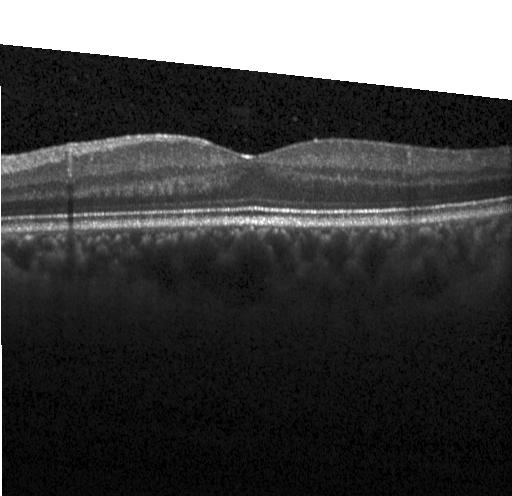
Finding: no evidence of choroidal neovascularization, diabetic macular edema, or drusen.